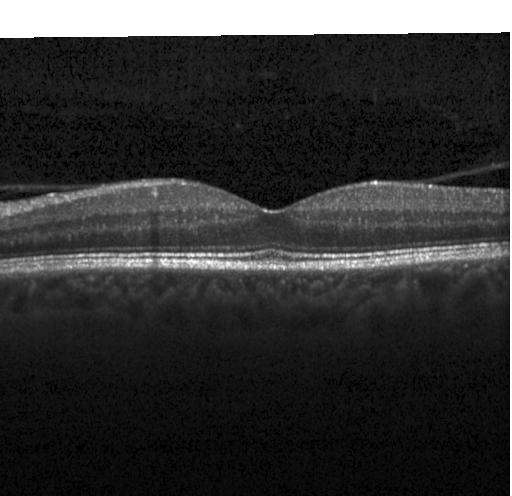
Neither choroidal neovascularization, diabetic macular edema, nor drusen.